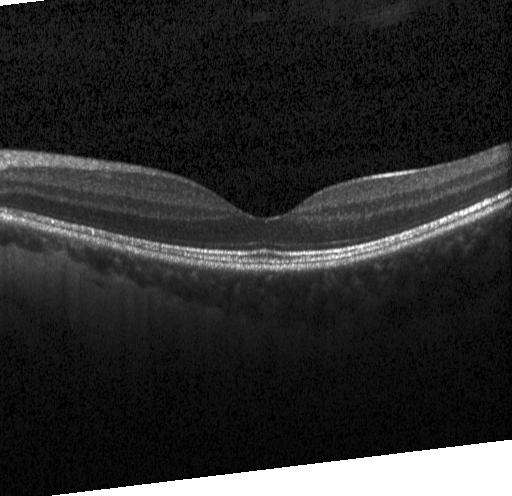 Optical coherence tomography scan. SD-OCT. Acquired on a Heidelberg Spectralis
Finding: no choroidal neovascularization, diabetic macular edema, or drusen.